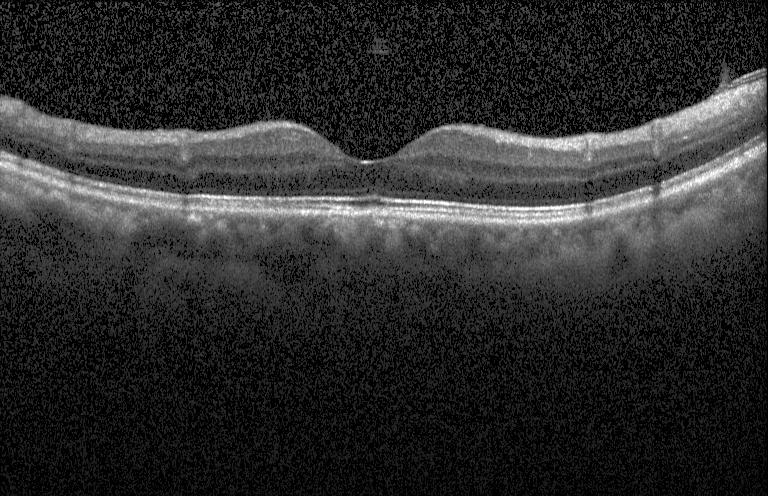 Horizontal scan through the fovea · SD-OCT · acquired on a Heidelberg Spectralis · optical coherence tomography scan — OCT finding: no CNV, DME, or drusen.